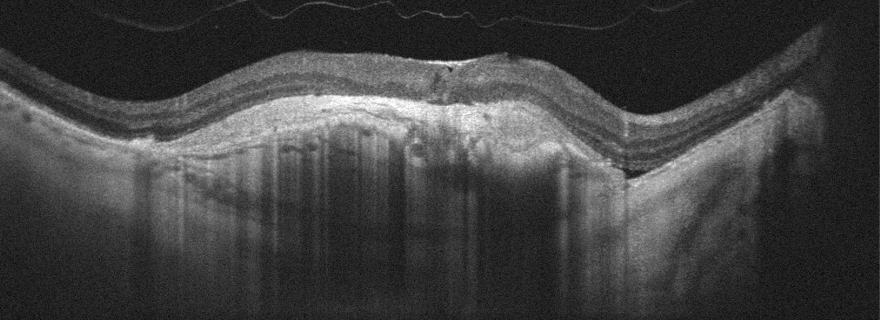
OCT line scan.
Diagnosis: AMD.